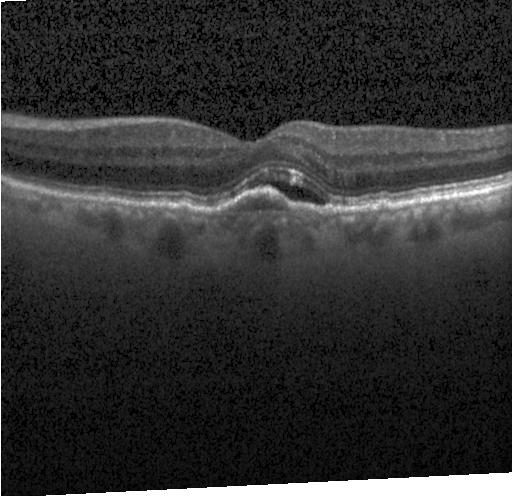 SD-OCT · Heidelberg Spectralis · OCT line scan · through the macula — Finding: a choroidal neovascular membrane.